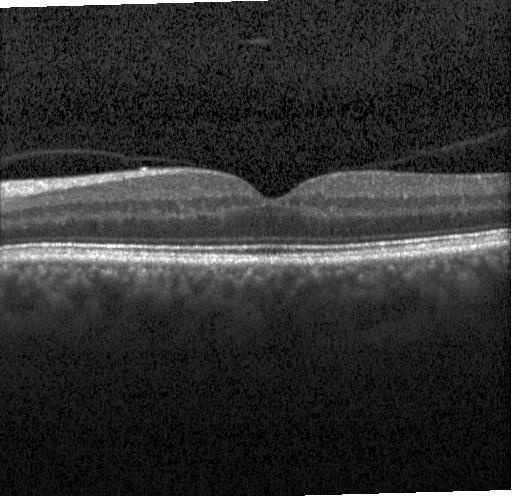 This B-scan demonstrates no evidence of choroidal neovascularization, diabetic macular edema, or drusen.